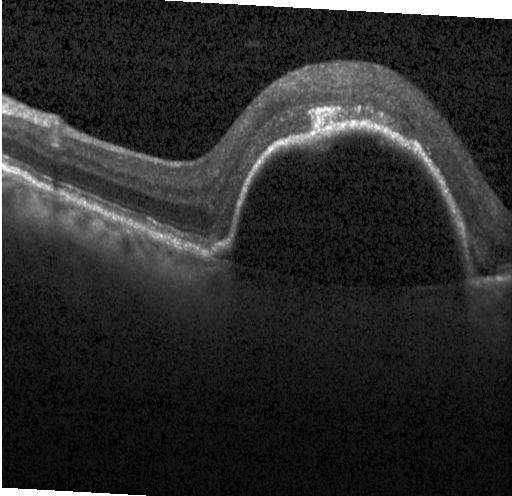

Finding: choroidal neovascularization (CNV).